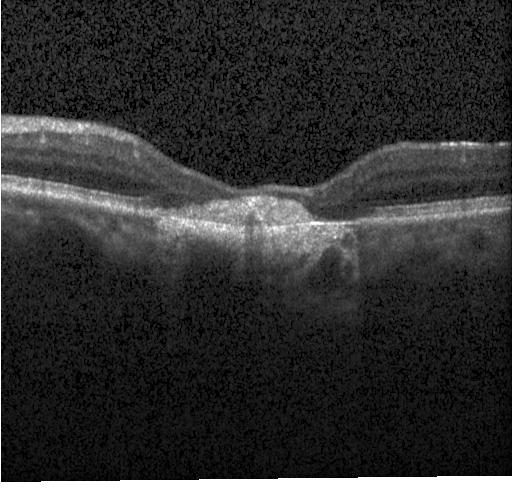
Dx: a choroidal neovascular membrane.